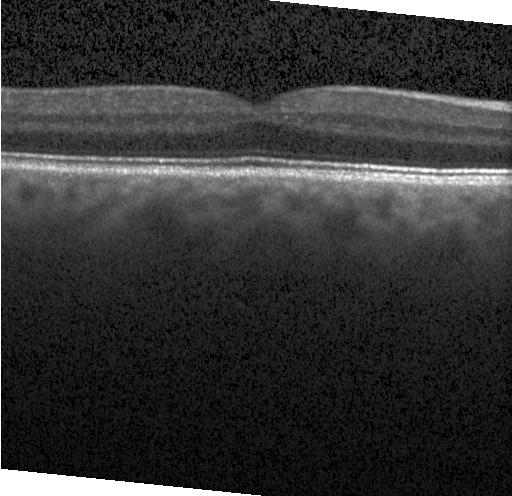
Heidelberg Spectralis OCT system · through the macula · spectral-domain optical coherence tomography · optical coherence tomography B-scan
Assessment: neither CNV, DME, nor drusen.